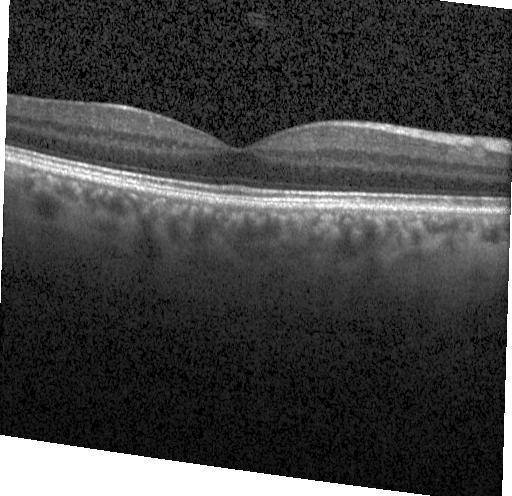
Optical coherence tomography B-scan · acquired on a Heidelberg Spectralis · macular scan. Macular OCT: no choroidal neovascularization, no diabetic macular edema, and no drusen.